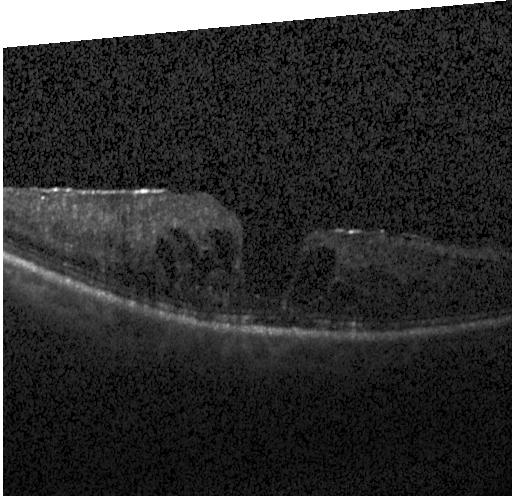
OCT B-scan showing diabetic macular edema.